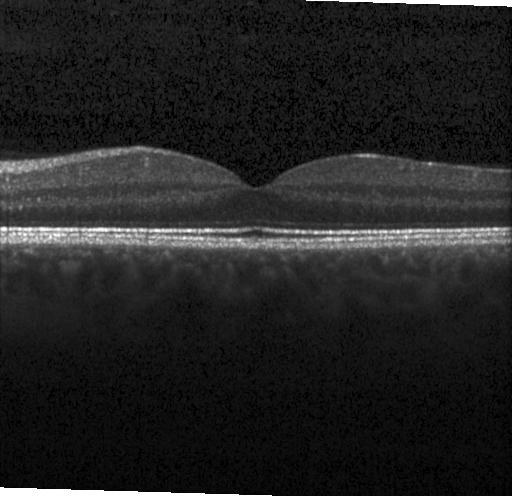 Finding: no CNV, DME, or drusen.